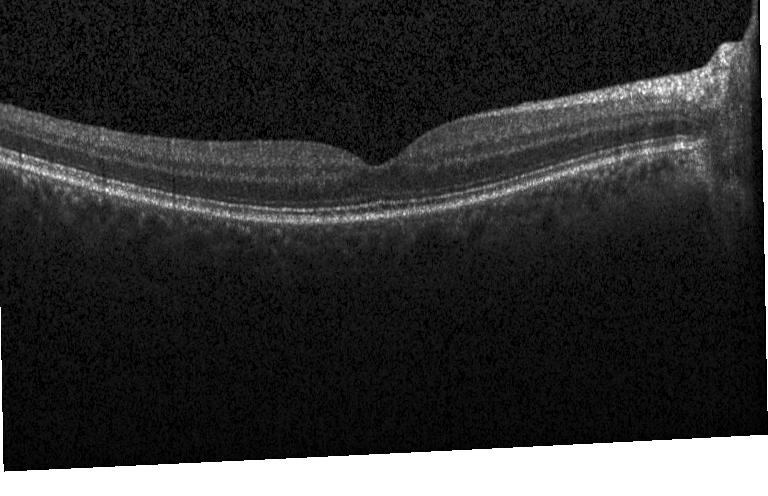 SD-OCT · centered on the fovea · Heidelberg Spectralis OCT system · optical coherence tomography B-scan
Impression: neither CNV, DME, nor drusen.